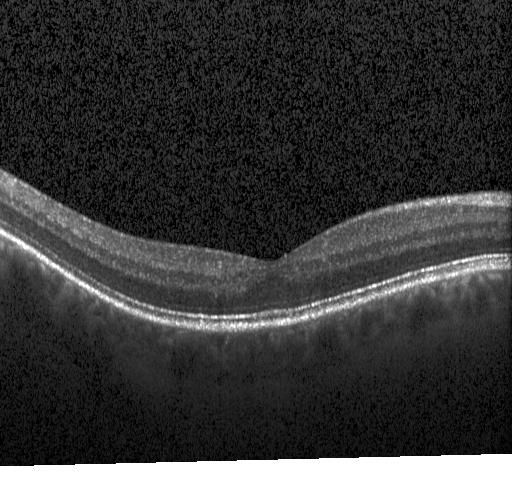 Optical coherence tomography scan, acquired on a Heidelberg Spectralis, SD-OCT. Diagnosis: no evidence of CNV, DME, or drusen.